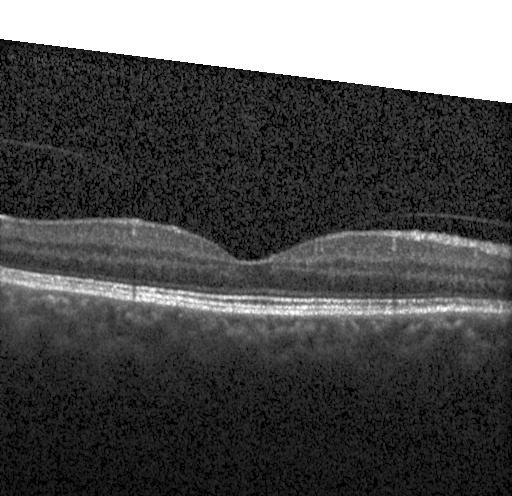

Through the macula; SD-OCT; retinal OCT B-scan
Finding: neither choroidal neovascularization, diabetic macular edema, nor drusen.